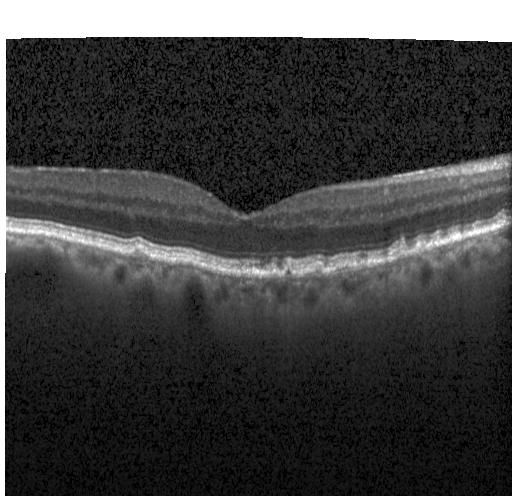 SD-OCT. Optical coherence tomography scan. Macular scan.
Impression: sub-RPE drusenoid deposits.